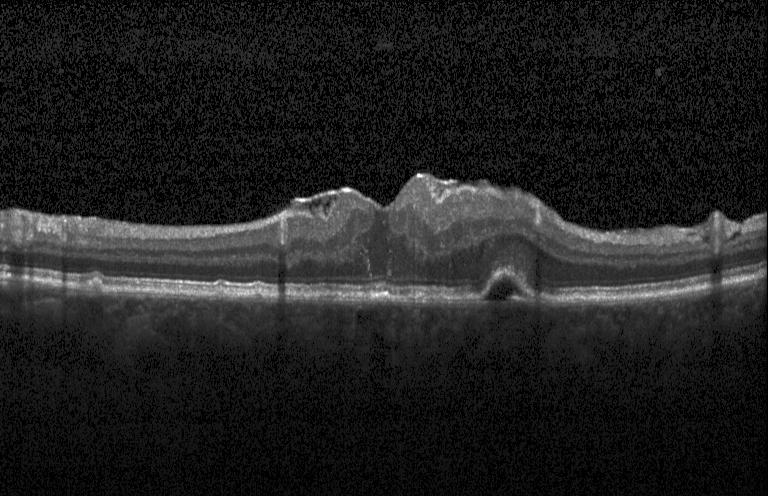

Retinal OCT B-scan. Macular scan. Heidelberg Spectralis
Impression: CNV.